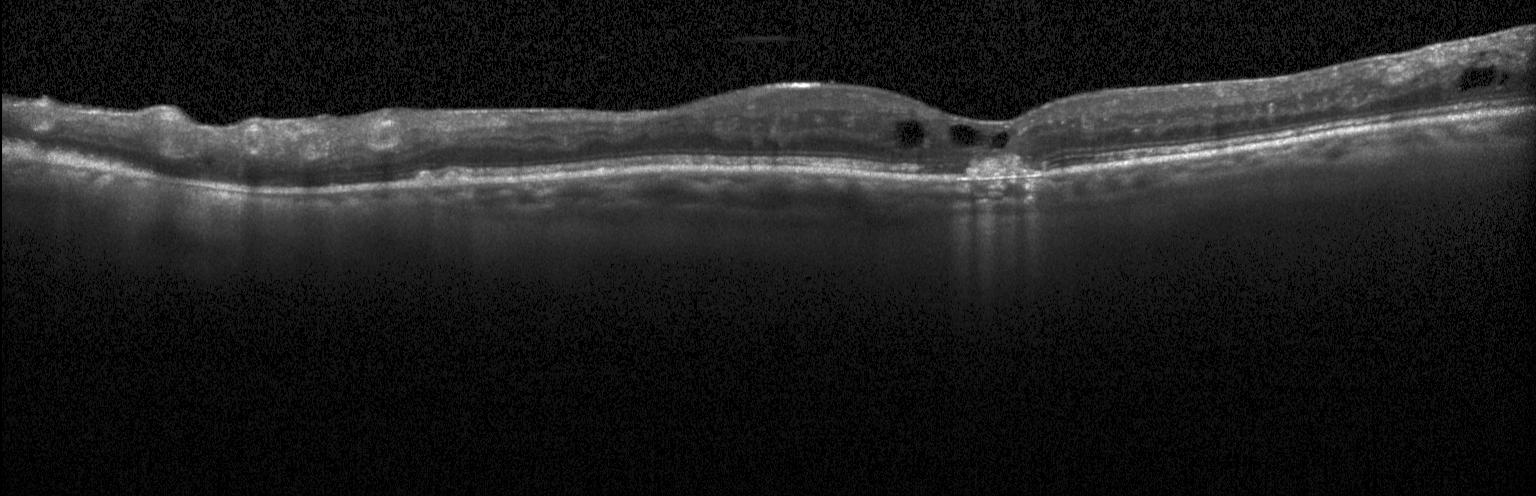

The scan shows a choroidal neovascular membrane.